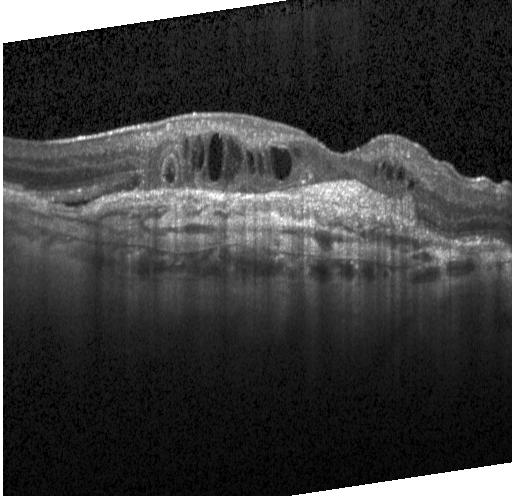
OCT line scan
A choroidal neovascular membrane.